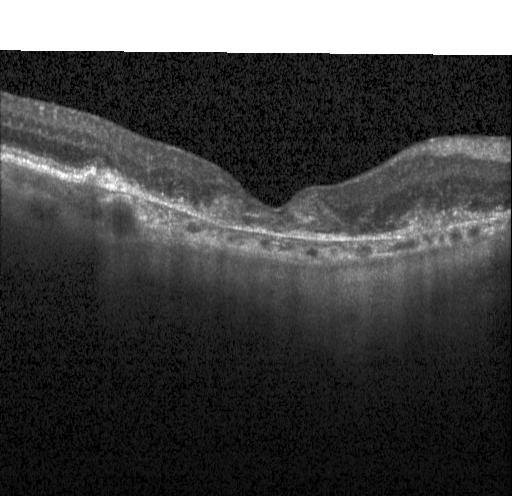 Finding: a choroidal neovascular membrane.